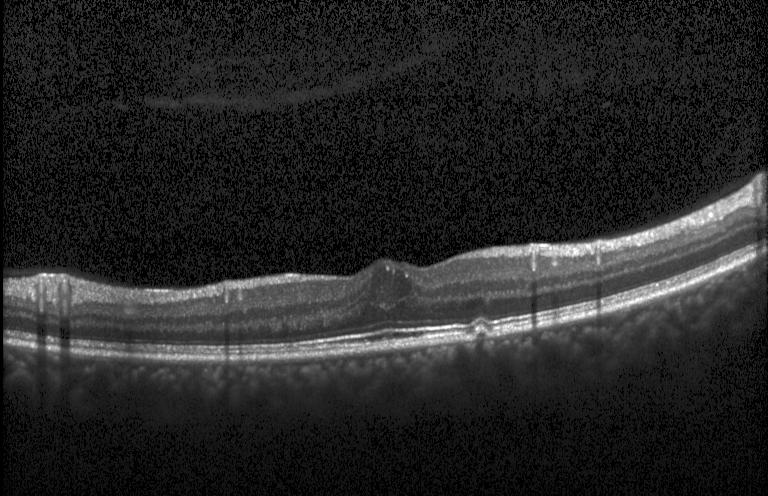
Centered on the fovea. Acquired on a Heidelberg Spectralis. Retinal OCT B-scan
Macular OCT: multiple drusen.